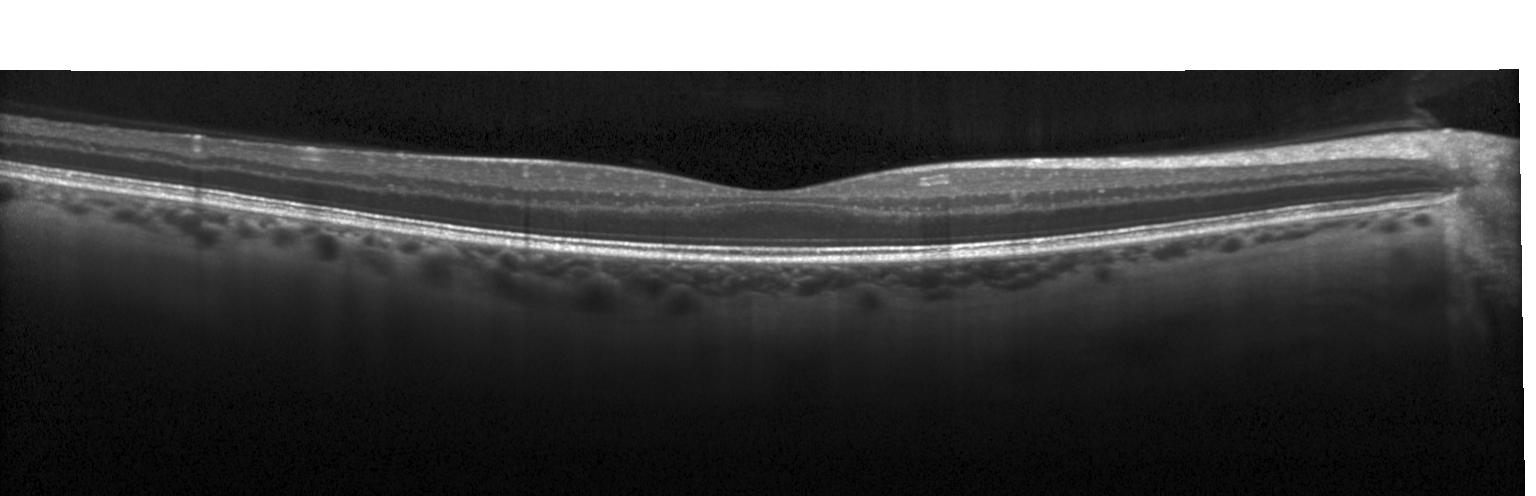
Impression: no CNV, DME, or drusen.